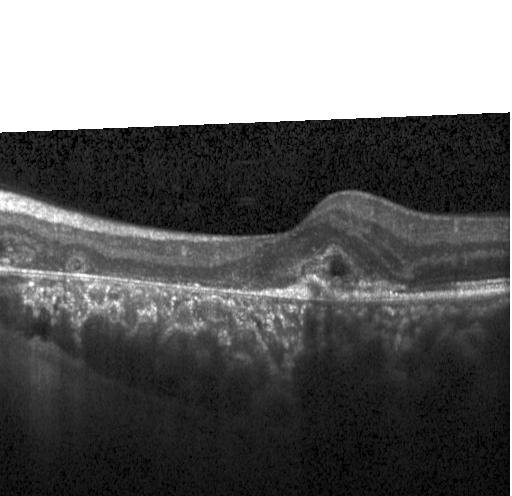 Retinal OCT cross-section showing a choroidal neovascular membrane.